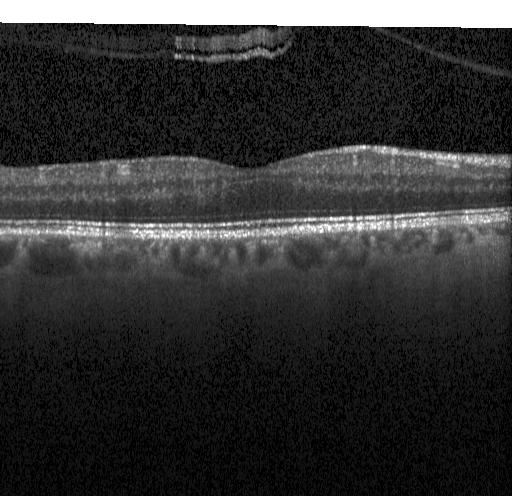 OCT B-scan. Impression: neither CNV, DME, nor drusen.